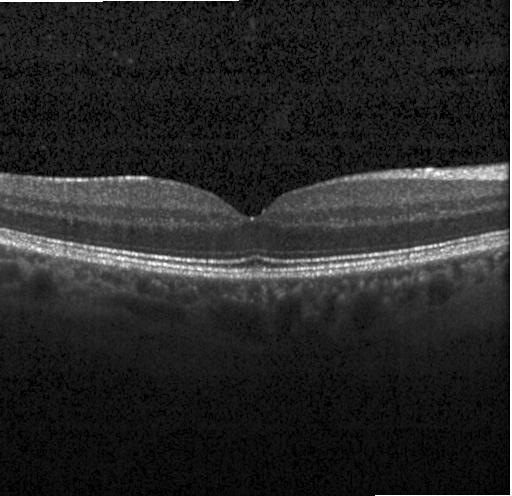
OCT finding: no evidence of CNV, DME, or drusen.